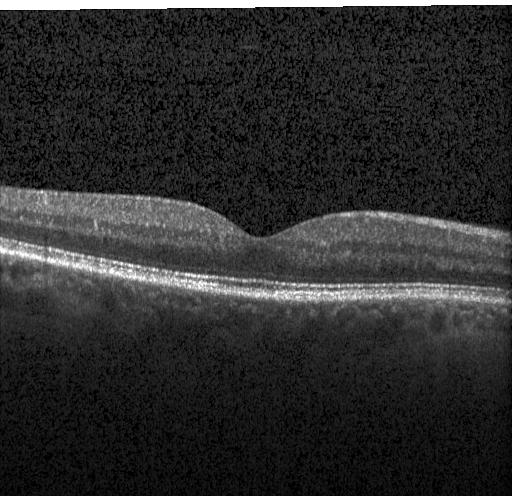
Centered on the fovea, spectral-domain optical coherence tomography, Heidelberg Spectralis, OCT B-scan. The scan shows no choroidal neovascularization, no diabetic macular edema, and no drusen.